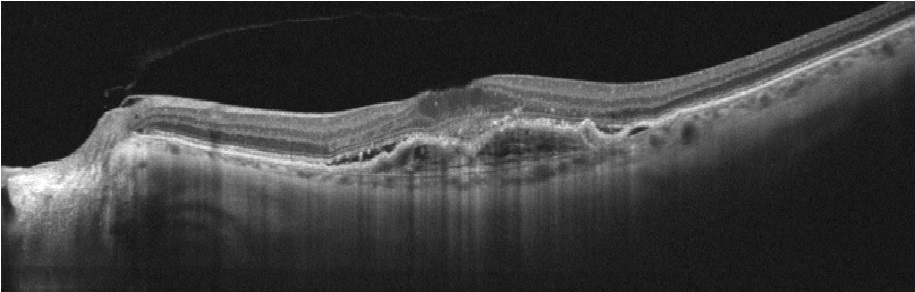 Optical coherence tomography scan. Diagnosis: age-related macular degeneration.